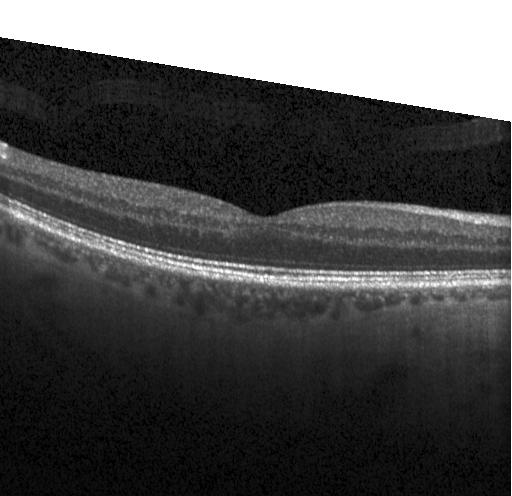 Acquired on a Heidelberg Spectralis; through the macula; optical coherence tomography B-scan
Diagnosis: neither CNV, DME, nor drusen.